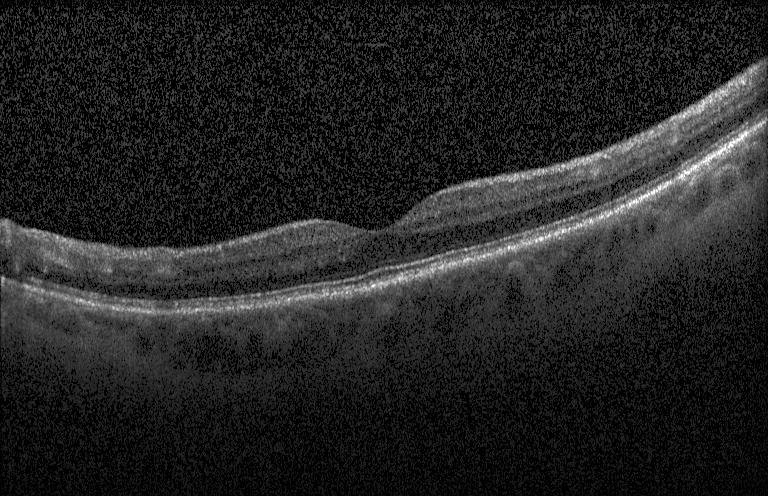

Retinal OCT B-scan — Finding: no choroidal neovascularization, diabetic macular edema, or drusen.